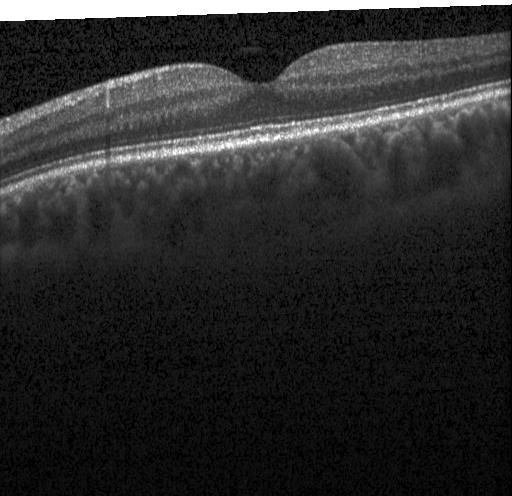 Finding: neither choroidal neovascularization, diabetic macular edema, nor drusen.